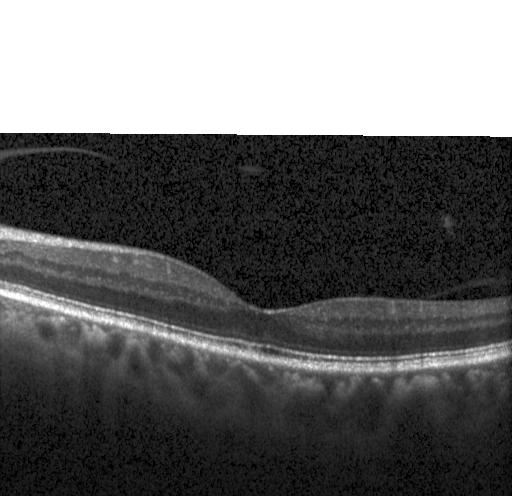

Diagnosis: neither choroidal neovascularization, diabetic macular edema, nor drusen.